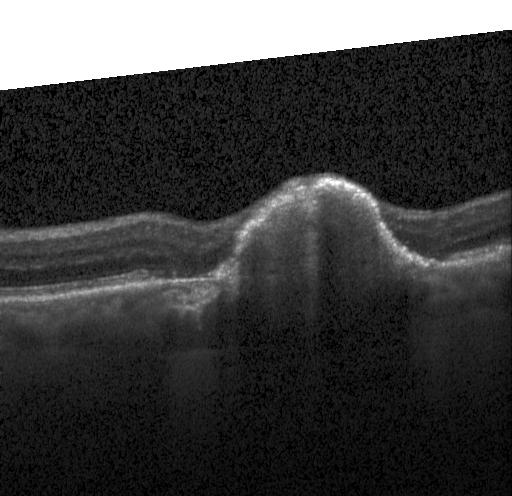
OCT line scan — OCT finding: choroidal neovascularization.